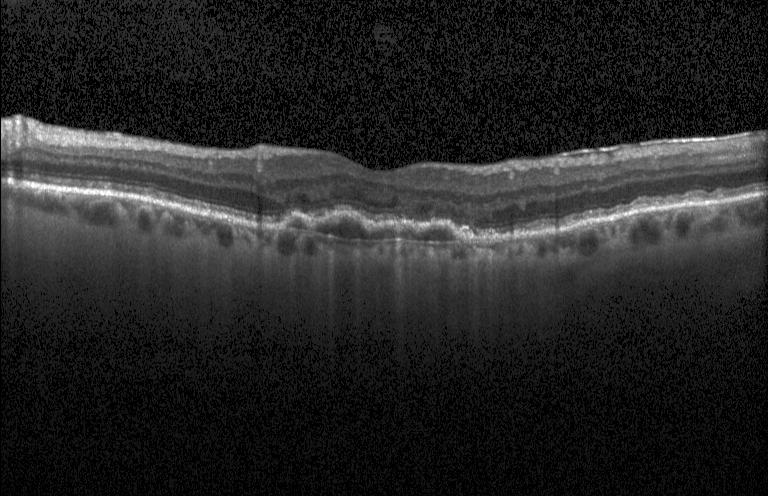
Impression: a choroidal neovascular membrane.